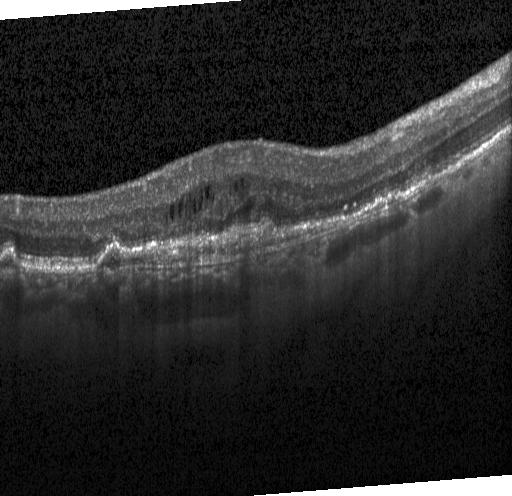
SD-OCT; instrument: Heidelberg Spectralis; horizontal scan through the fovea; OCT B-scan.
Macular OCT: a choroidal neovascular membrane.